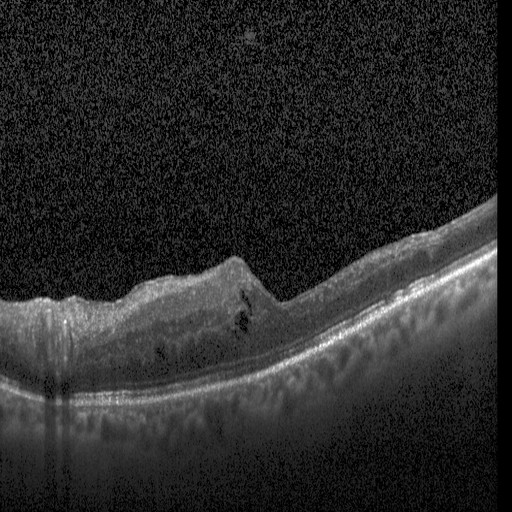 OCT B-scan. The scan shows diabetic macular edema.